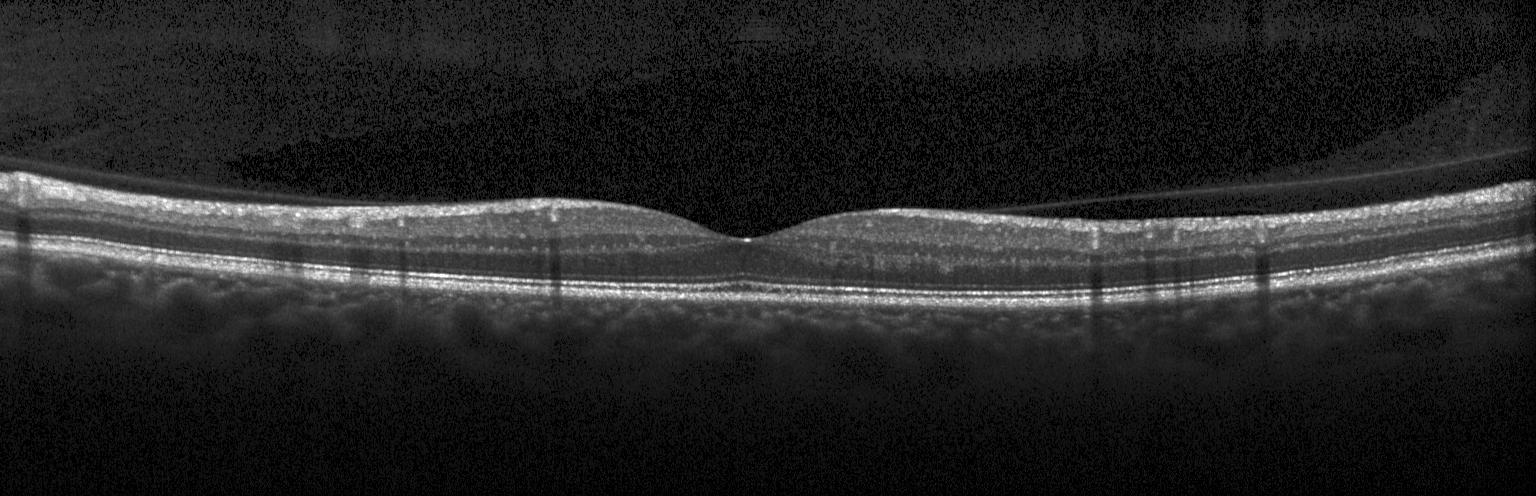 Optical coherence tomography scan, fovea-centered.
Impression: neither choroidal neovascularization, diabetic macular edema, nor drusen.